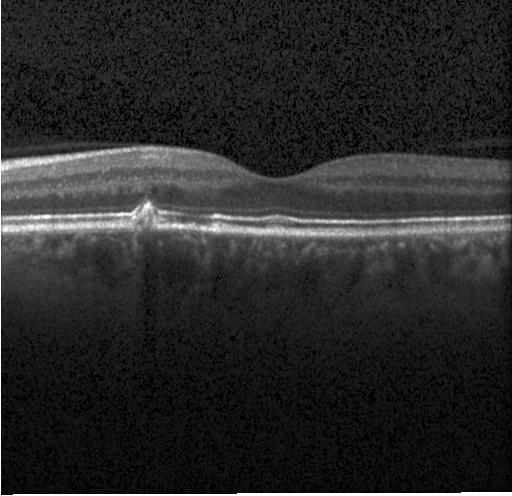

Spectral-domain OCT B-scan: drusen.